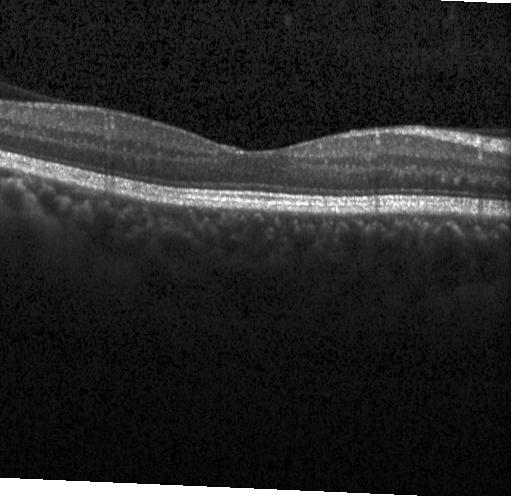 Retinal OCT B-scan. Assessment: no choroidal neovascularization, diabetic macular edema, or drusen.